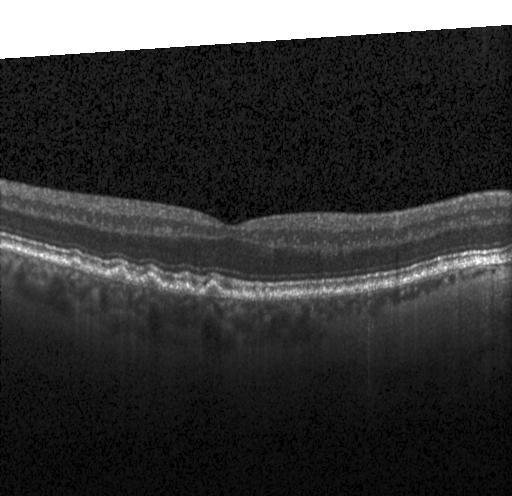
Spectral-domain optical coherence tomography · through the macula · Heidelberg Spectralis · OCT line scan
Assessment: sub-RPE drusenoid deposits.